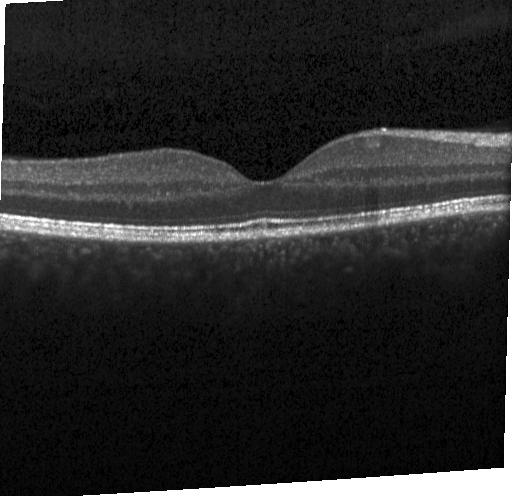 Optical coherence tomography B-scan
The scan shows no CNV, no DME, and no drusen.